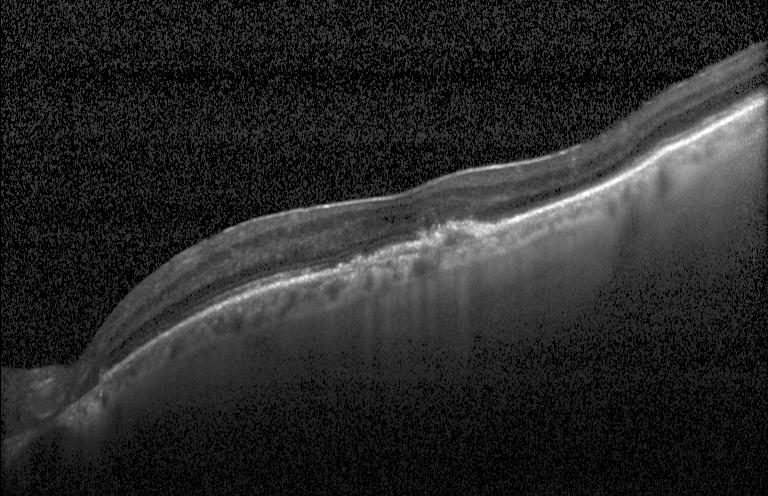 Macular scan, OCT line scan. Finding: choroidal neovascularization.